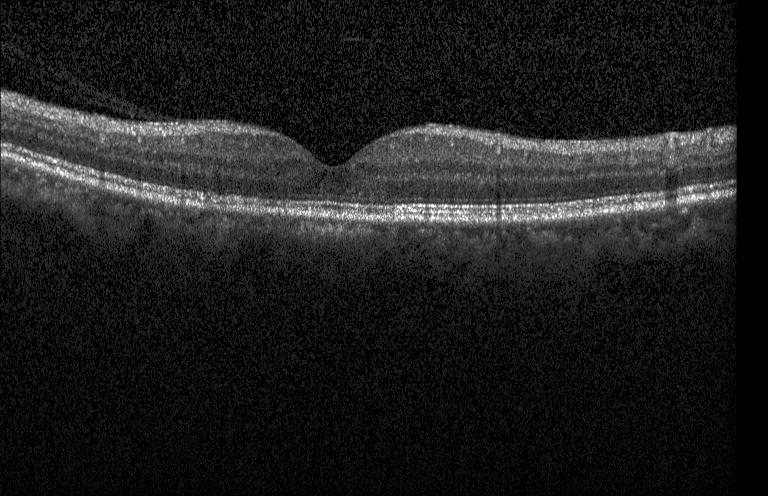 Optical coherence tomography B-scan.
The scan shows neither choroidal neovascularization, diabetic macular edema, nor drusen.